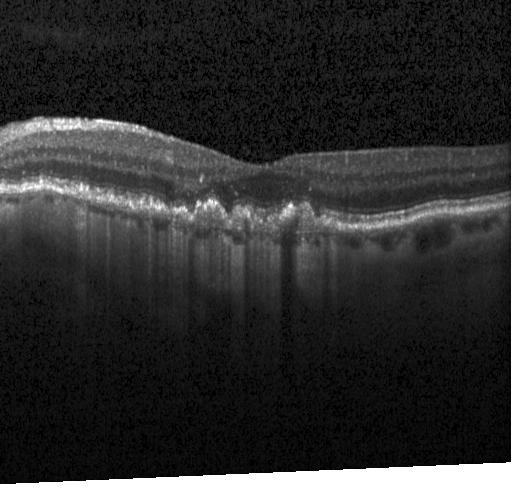
The scan shows drusen.